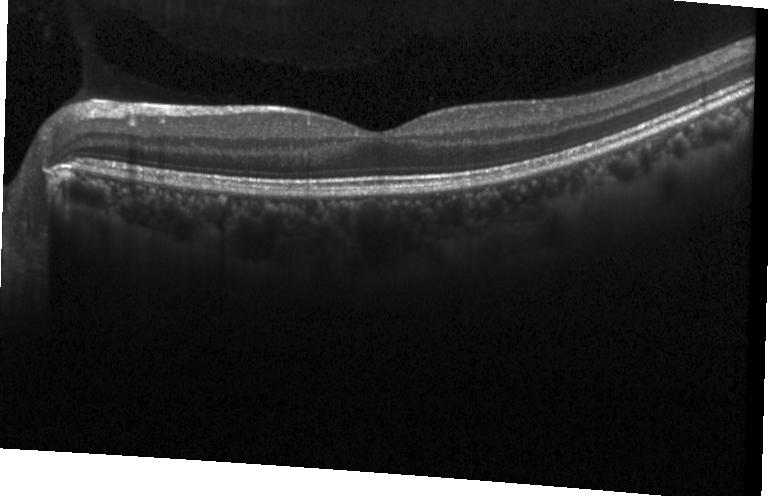

OCT B-scan showing no evidence of CNV, DME, or drusen.